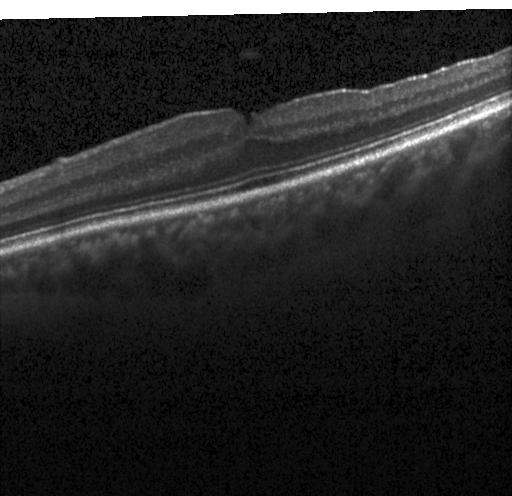
Retinal OCT B-scan. Impression: no evidence of CNV, DME, or drusen.